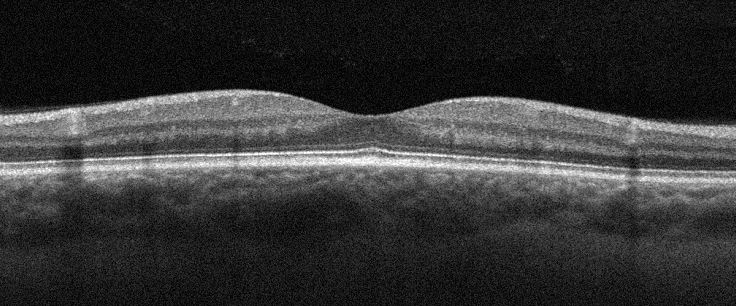

Macular OCT demonstrating no evidence of AMD, DME, ERM, RAO, RVO, or VID.